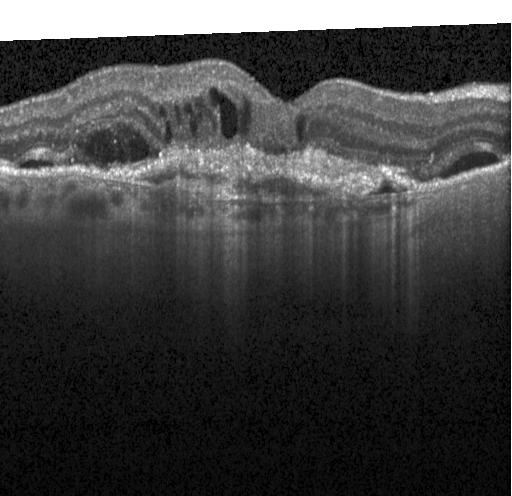
OCT finding: a choroidal neovascular membrane.